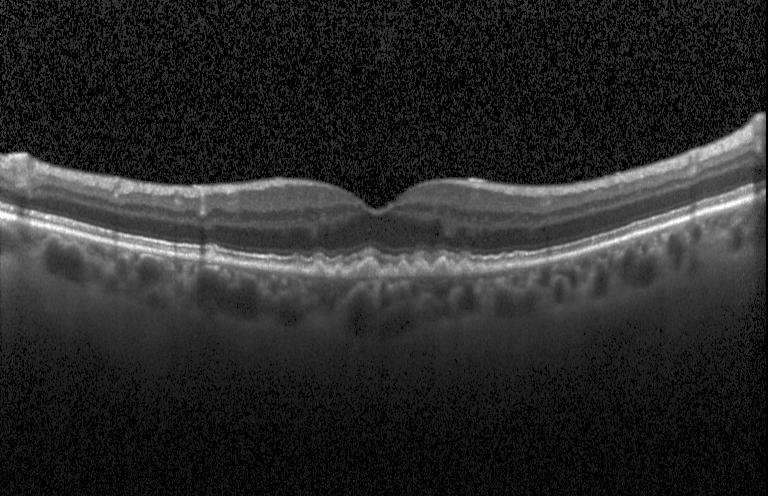
Macular OCT demonstrating drusen.